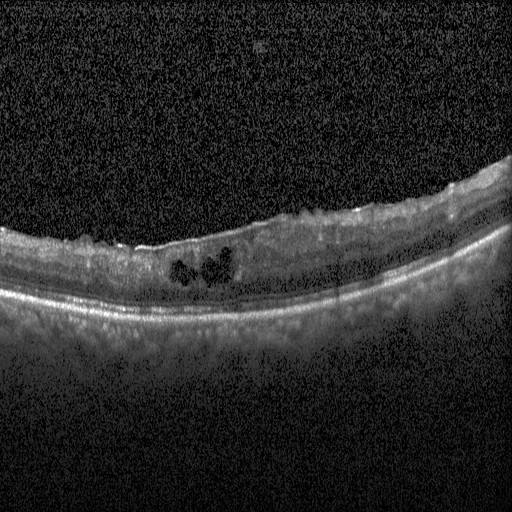
Impression: diabetic macular edema (DME).